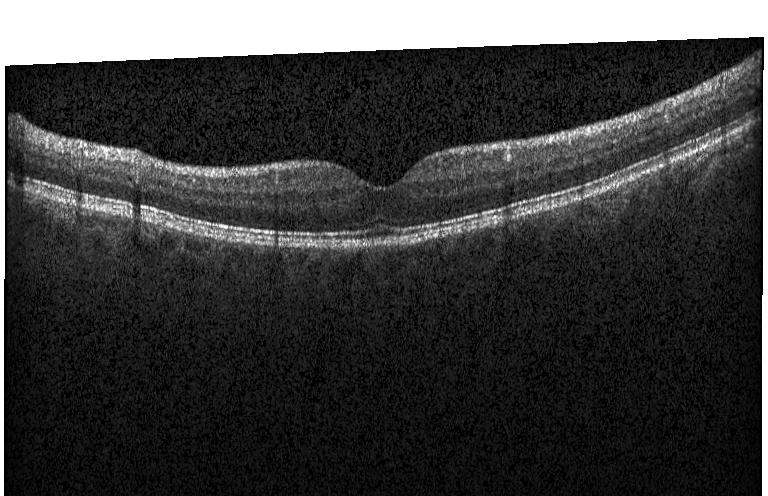
SD-OCT. Through the macula. Instrument: Heidelberg Spectralis. Retinal OCT B-scan — Impression: neither choroidal neovascularization, diabetic macular edema, nor drusen.